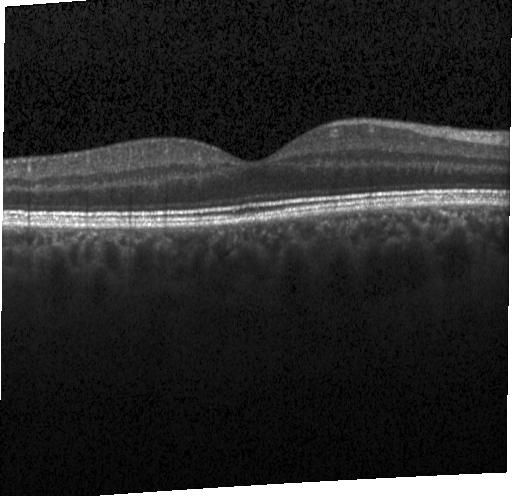

Optical coherence tomography scan — Macular OCT: no evidence of choroidal neovascularization, diabetic macular edema, or drusen.